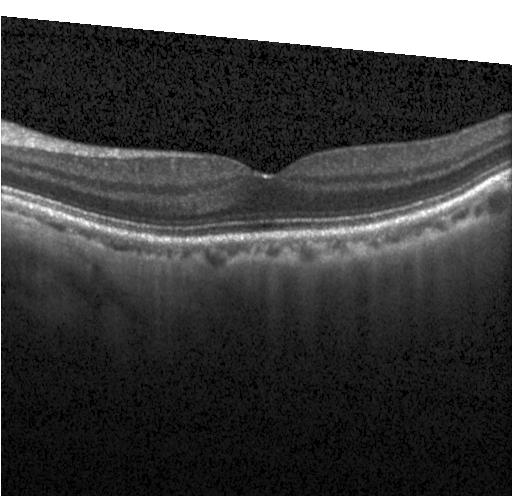

Diagnosis: no evidence of choroidal neovascularization, diabetic macular edema, or drusen.